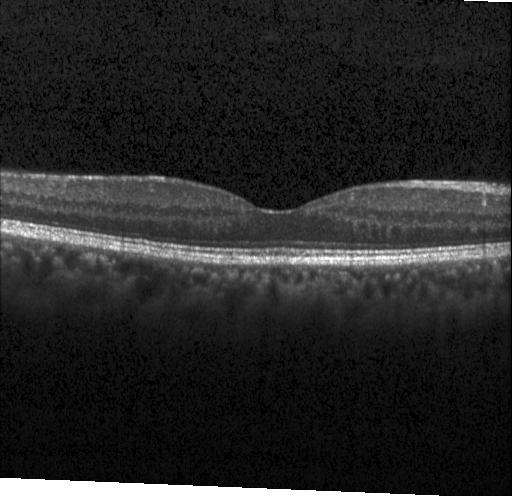 The scan shows no CNV, DME, or drusen.